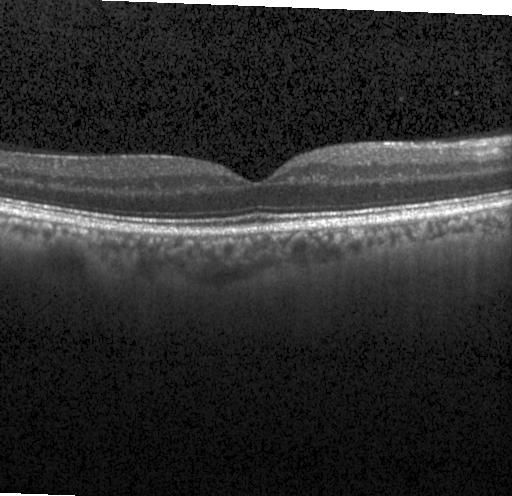

Retinal OCT cross-section showing no choroidal neovascularization, no diabetic macular edema, and no drusen.